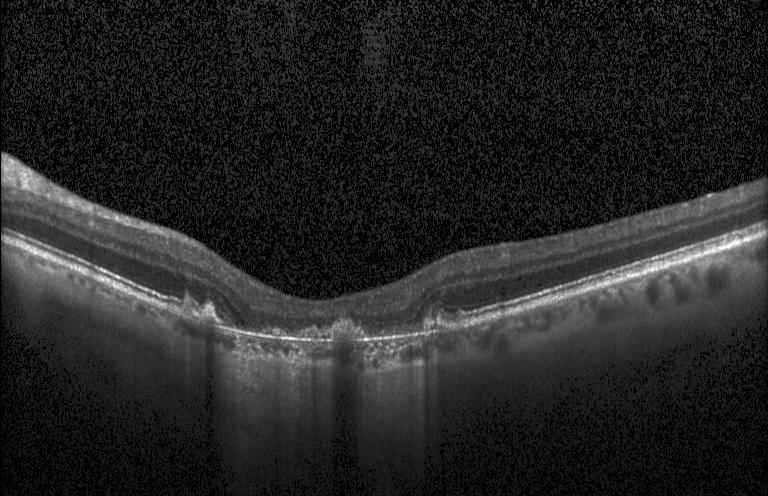
Heidelberg Spectralis OCT system; macular scan; SD-OCT; retinal OCT cross-section.
Diagnosis: a choroidal neovascular membrane.